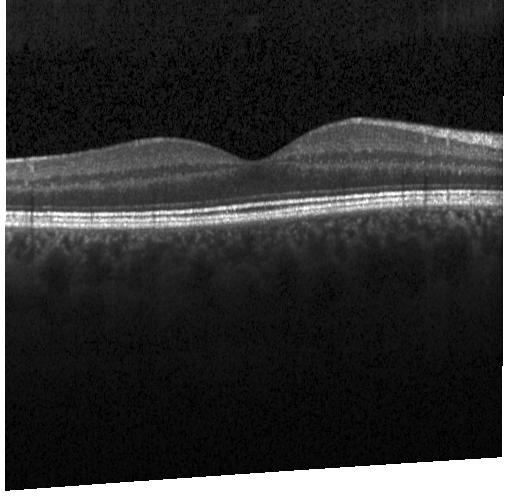 Diagnosis: no choroidal neovascularization, no diabetic macular edema, and no drusen.